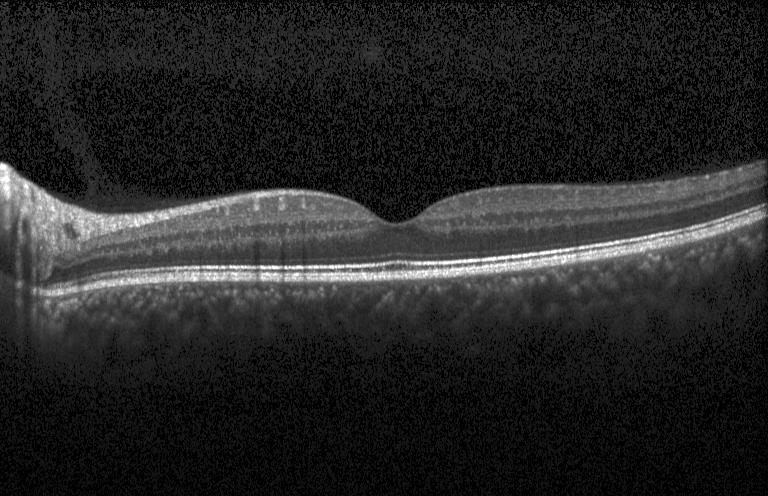 Diagnosis: no choroidal neovascularization, diabetic macular edema, or drusen.